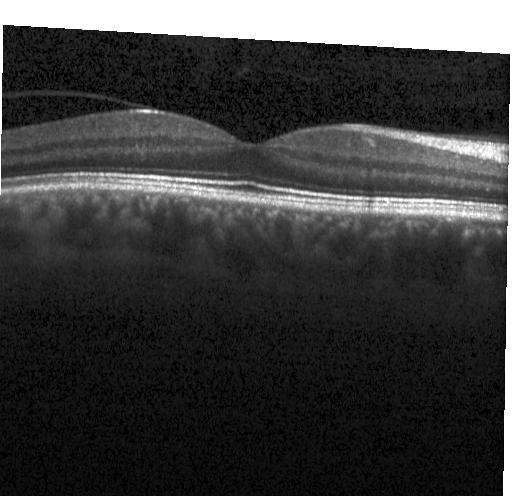
No evidence of choroidal neovascularization, diabetic macular edema, or drusen.